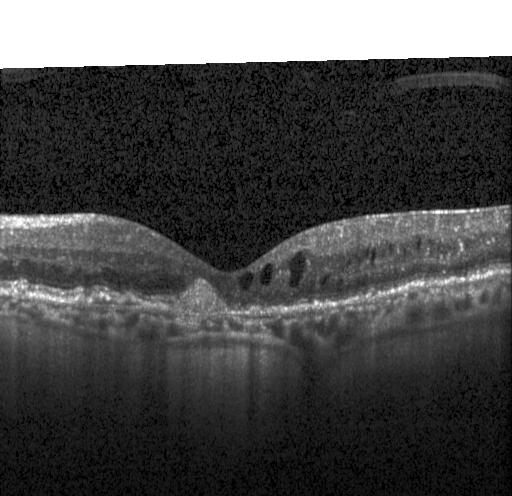 OCT finding: CNV.